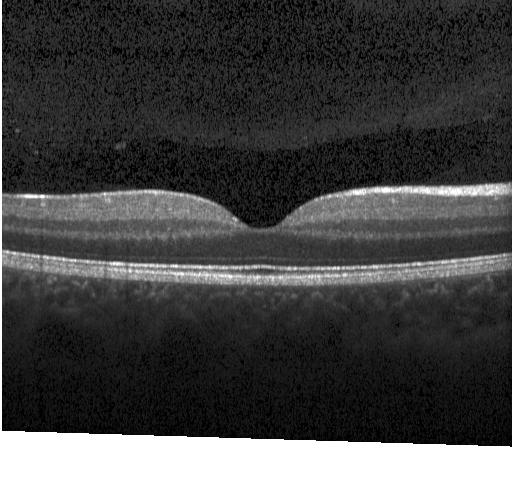 OCT scan showing no evidence of choroidal neovascularization, diabetic macular edema, or drusen.